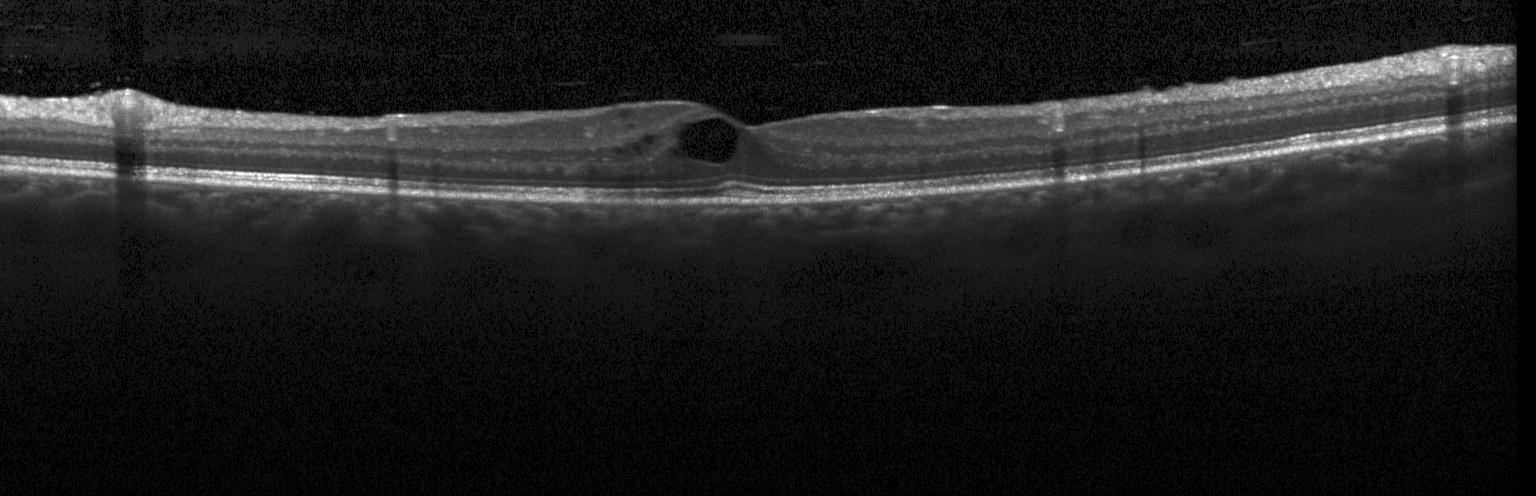
OCT B-scan · SD-OCT · through the macula.
Diagnosis: diabetic macular edema.